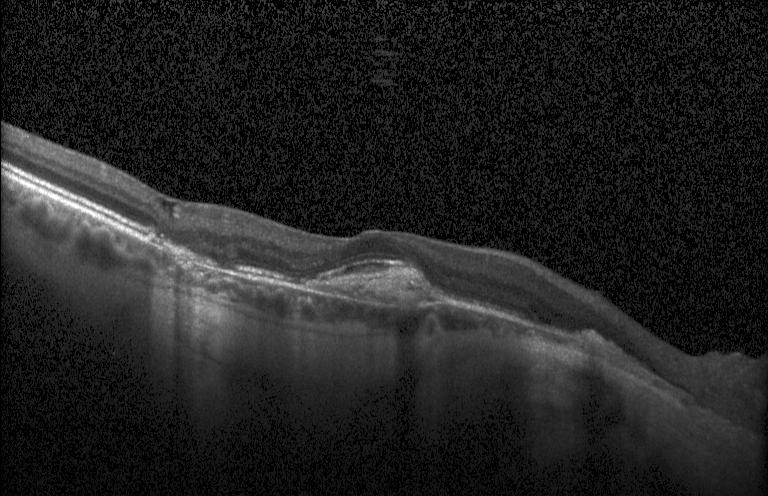 Centered on the fovea. Optical coherence tomography scan. Assessment: a choroidal neovascular membrane.